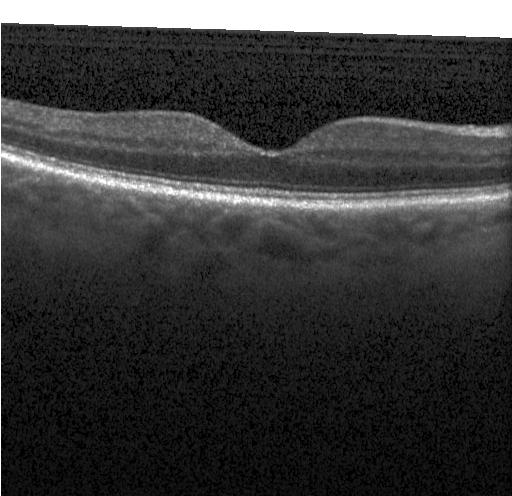 Spectral-domain optical coherence tomography. Acquired on a Heidelberg Spectralis. OCT line scan. Fovea-centered.
This B-scan demonstrates no evidence of choroidal neovascularization, diabetic macular edema, or drusen.